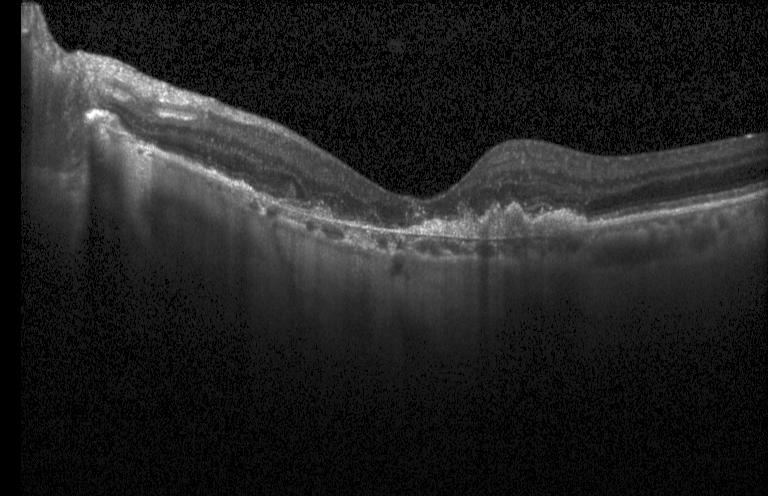
Retinal OCT B-scan. Spectral-domain optical coherence tomography. Heidelberg Spectralis.
OCT finding: choroidal neovascularization.